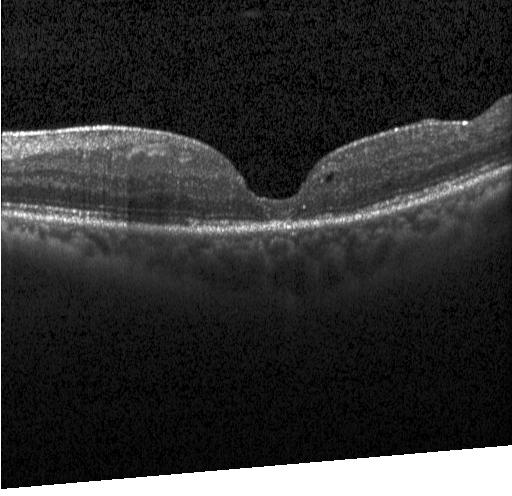 Spectral-domain OCT, instrument: Heidelberg Spectralis, OCT B-scan, macular scan.
Dx: diabetic macular edema (DME).